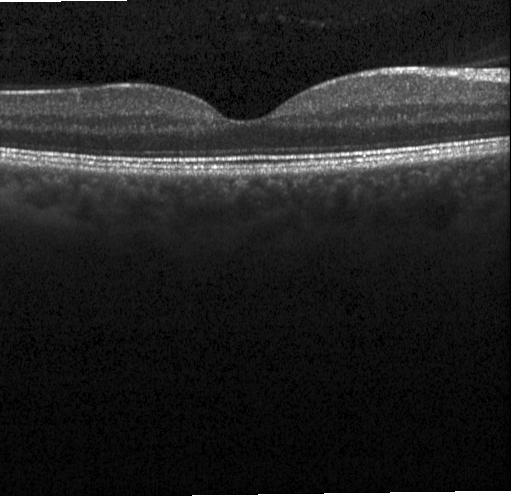 Finding: neither choroidal neovascularization, diabetic macular edema, nor drusen.